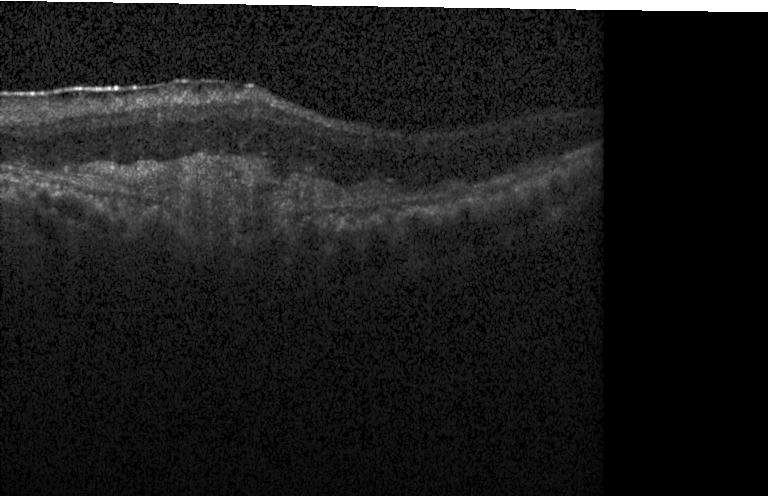
OCT line scan, Heidelberg Spectralis, macular scan, spectral-domain OCT.
Assessment: choroidal neovascularization (CNV).